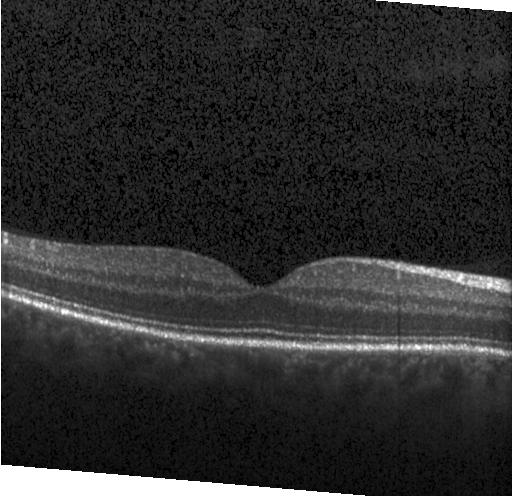
Retinal OCT cross-section · acquired on a Heidelberg Spectralis.
The scan shows no choroidal neovascularization, no diabetic macular edema, and no drusen.